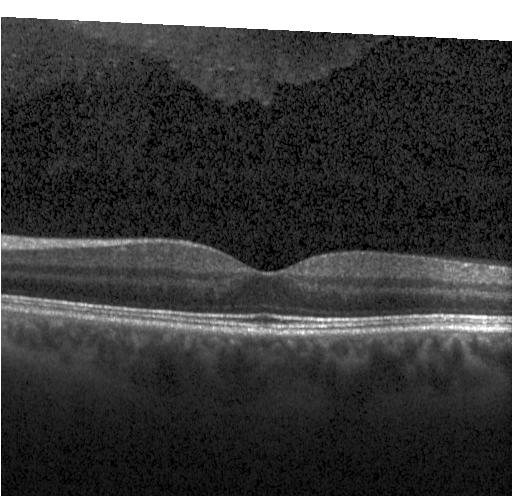 OCT B-scan — Impression: neither choroidal neovascularization, diabetic macular edema, nor drusen.